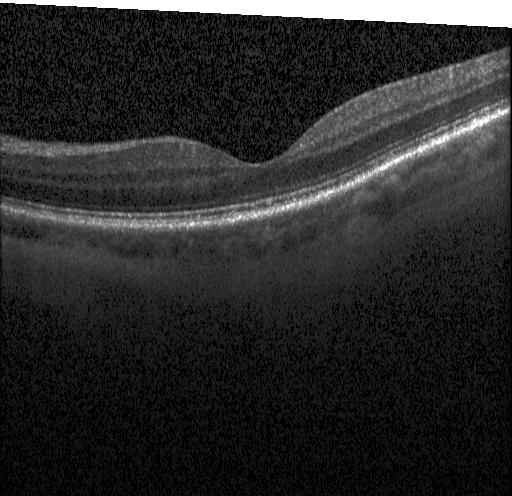 Spectral-domain OCT; centered on the fovea; optical coherence tomography B-scan
The scan shows no CNV, no DME, and no drusen.